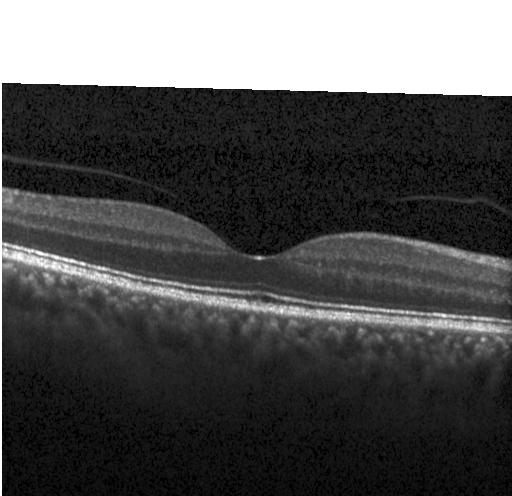
Retinal OCT B-scan
Diagnosis: no CNV, no DME, and no drusen.